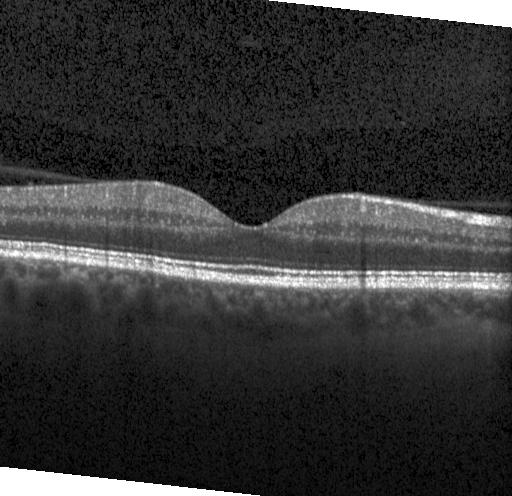
Heidelberg Spectralis; OCT B-scan.
Assessment: neither choroidal neovascularization, diabetic macular edema, nor drusen.